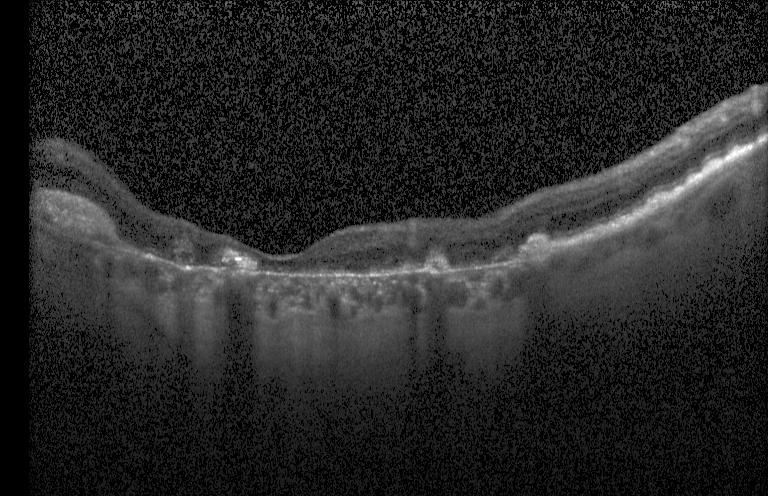 Impression: choroidal neovascularization.